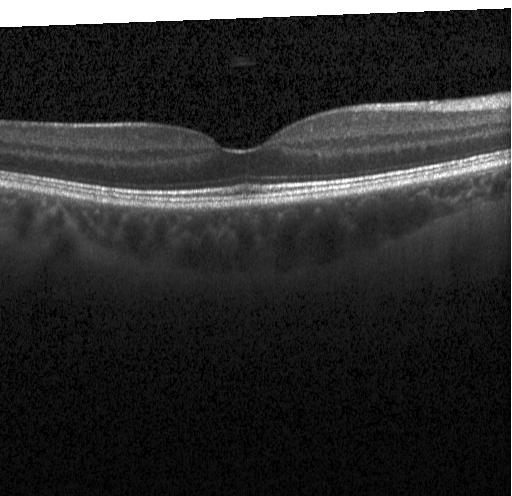 Retinal OCT B-scan; macular scan; instrument: Heidelberg Spectralis; spectral-domain OCT. Finding: no choroidal neovascularization, no diabetic macular edema, and no drusen.